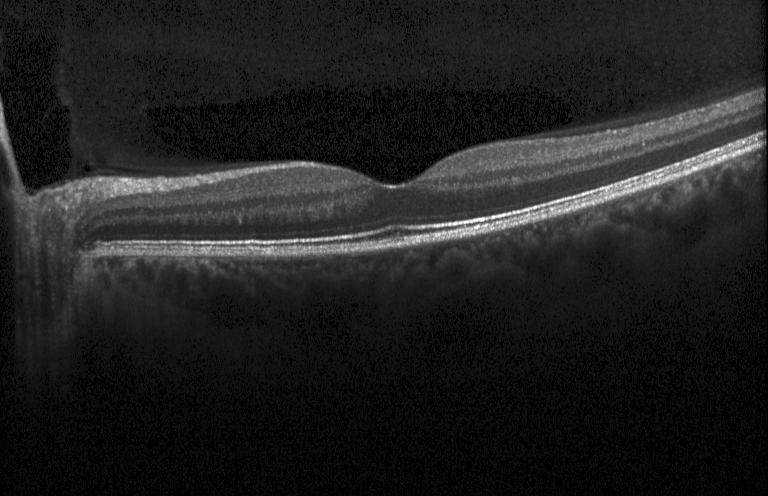

No CNV, DME, or drusen.